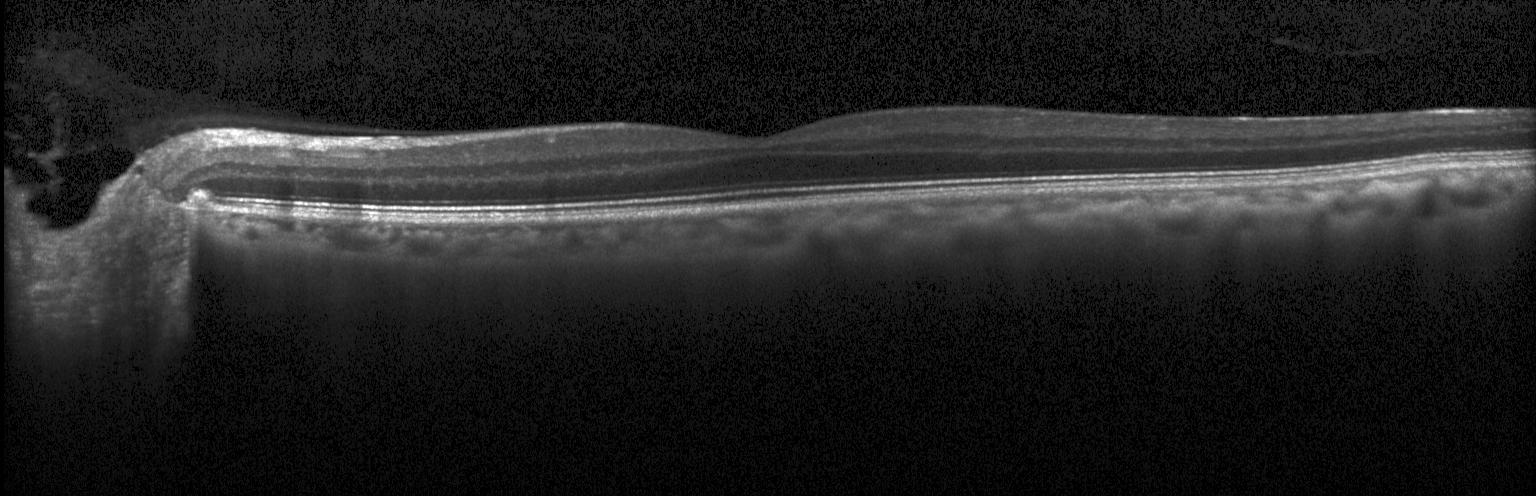

Heidelberg Spectralis OCT system, optical coherence tomography B-scan. Impression: no choroidal neovascularization, diabetic macular edema, or drusen.